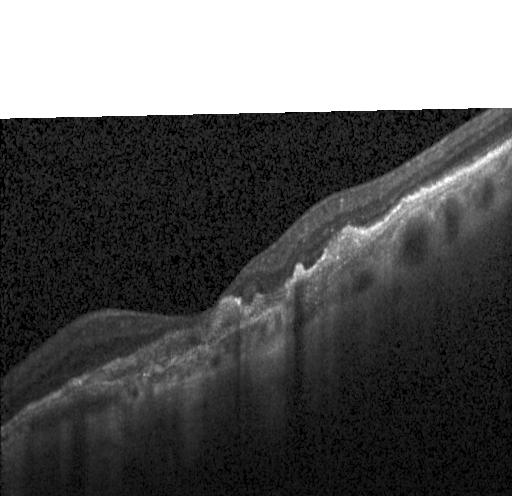 Optical coherence tomography scan — OCT finding: a choroidal neovascular membrane.